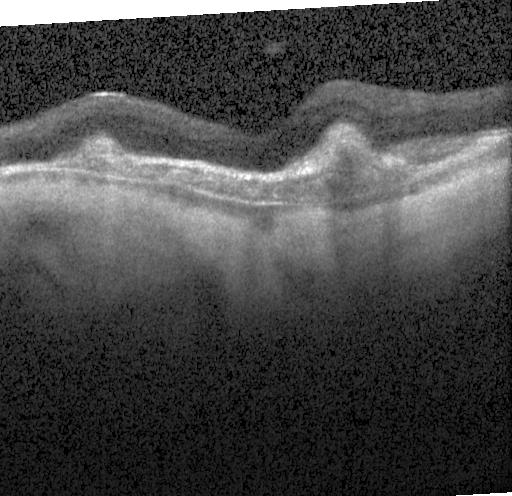

Diagnosis: CNV.